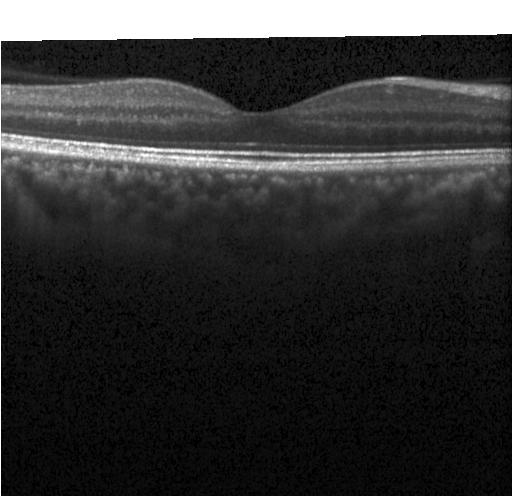
OCT line scan. OCT finding: no choroidal neovascularization, no diabetic macular edema, and no drusen.